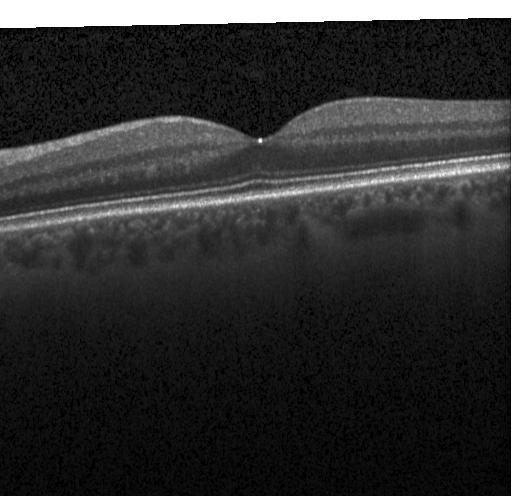
Spectral-domain OCT; optical coherence tomography scan.
Finding: no choroidal neovascularization, diabetic macular edema, or drusen.